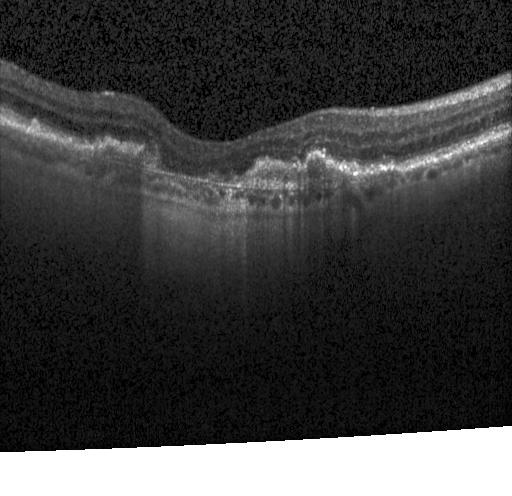 Macular OCT: a choroidal neovascular membrane.